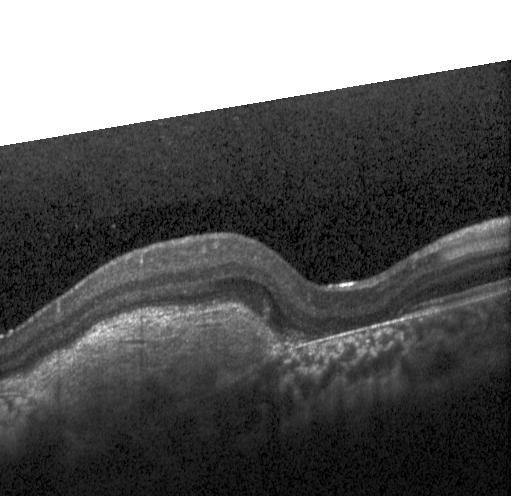
Finding: a choroidal neovascular membrane.